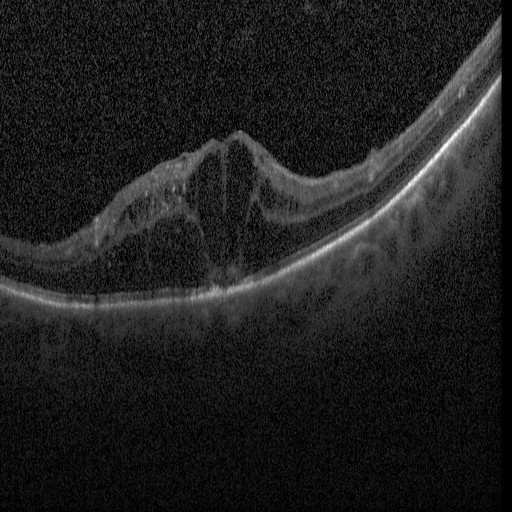 Spectral-domain OCT, Heidelberg Spectralis OCT system, retinal OCT B-scan, macular scan — Diagnosis: diabetic macular edema (DME).